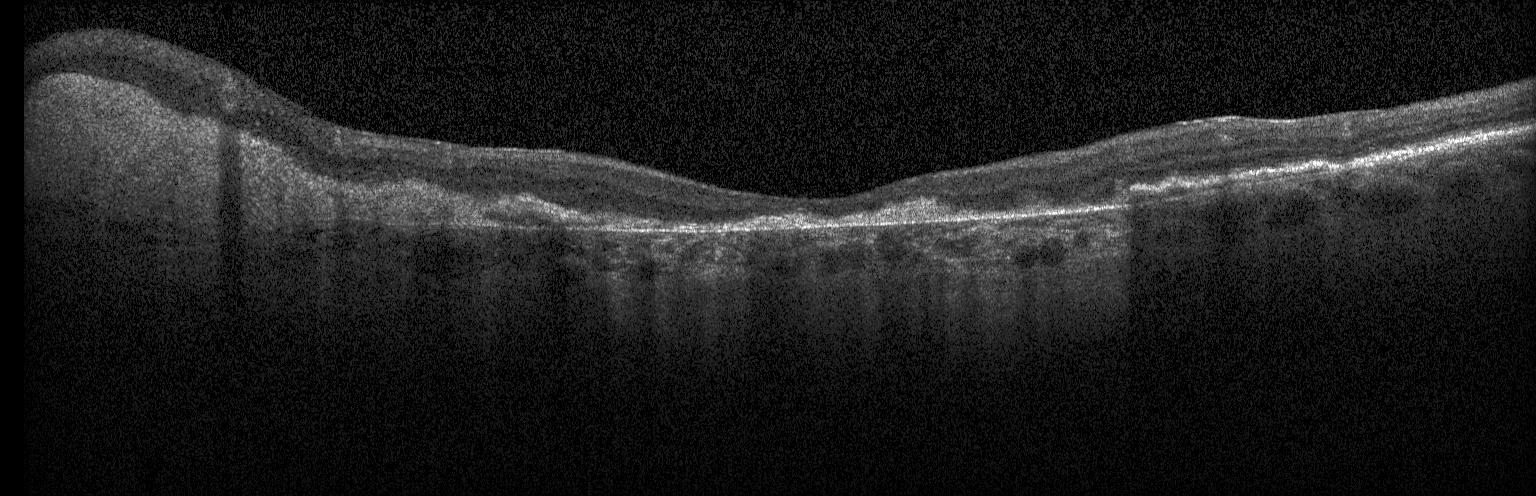 Acquired on a Heidelberg Spectralis · horizontal scan through the fovea · spectral-domain optical coherence tomography · optical coherence tomography scan — Assessment: choroidal neovascularization.